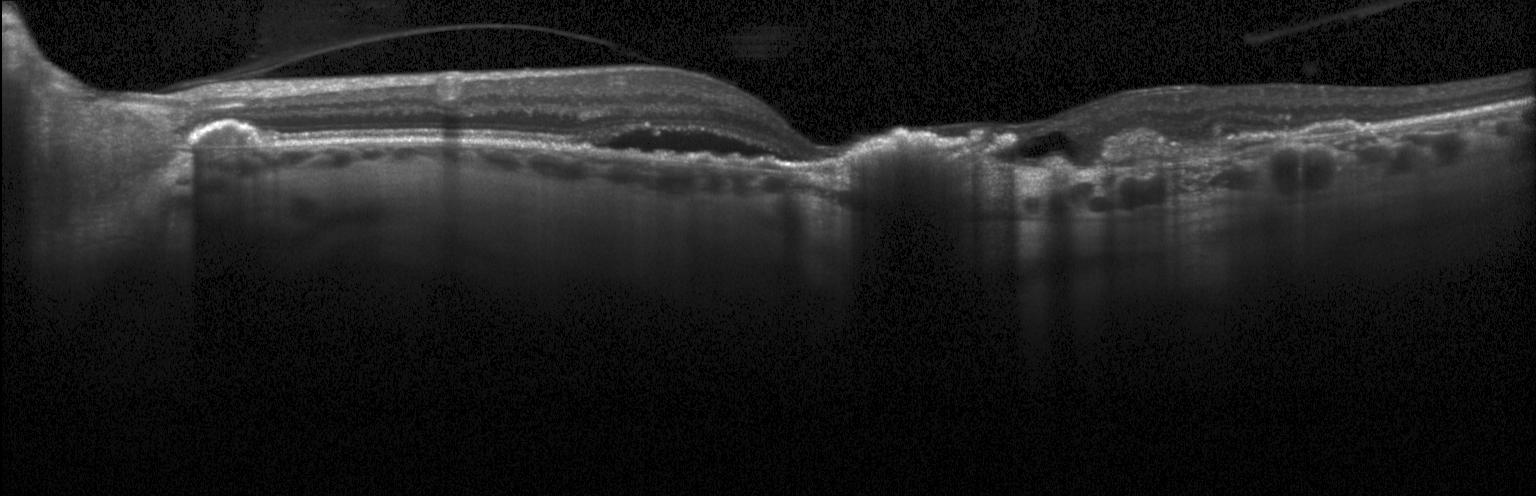

Optical coherence tomography scan · through the macula · Heidelberg Spectralis OCT system
Dx: CNV.